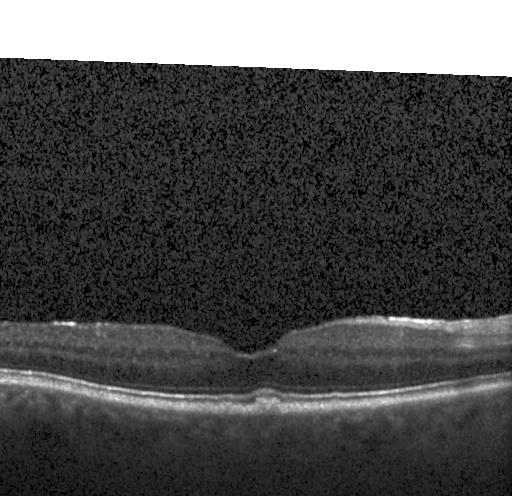
Heidelberg Spectralis OCT system · through the macula · SD-OCT · retinal OCT B-scan. The scan shows drusen.